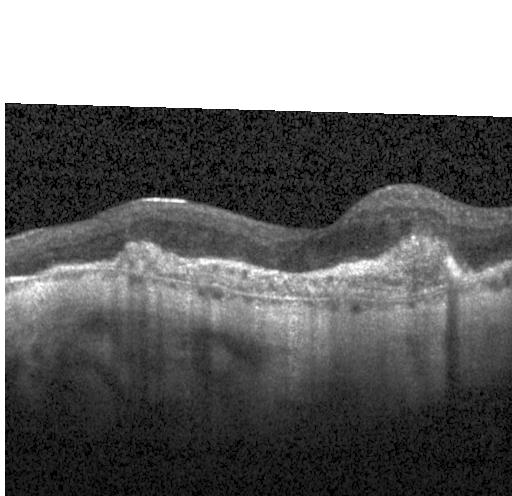 Diagnosis: a choroidal neovascular membrane.